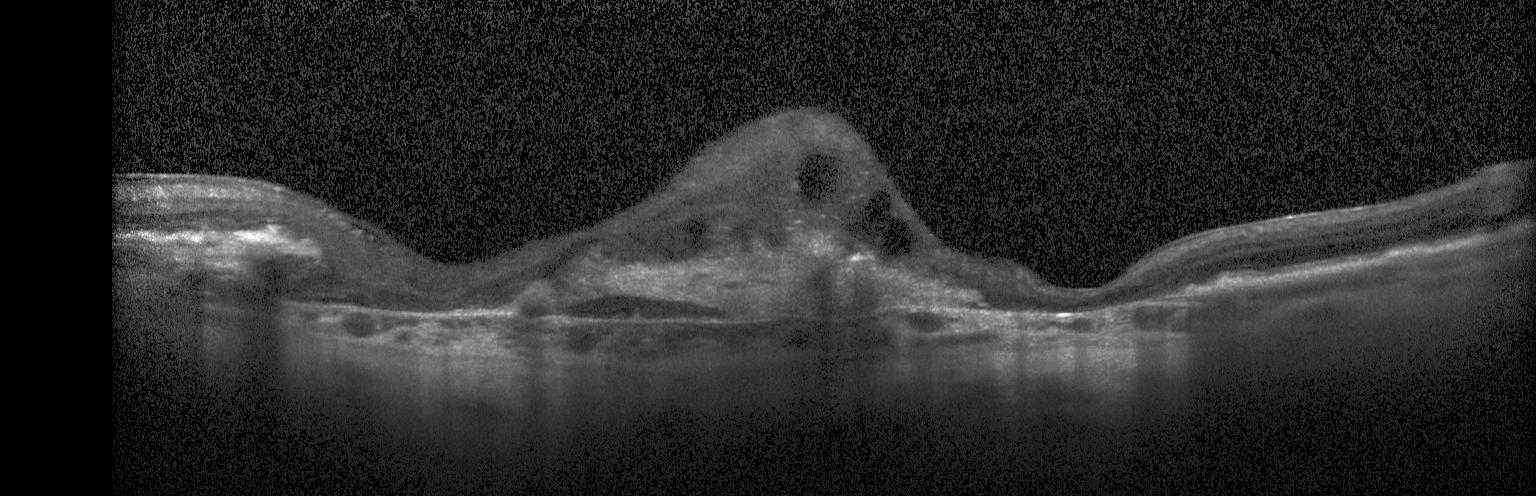

Retinal OCT B-scan · SD-OCT · Heidelberg Spectralis · macular scan — Macular OCT: a choroidal neovascular membrane.